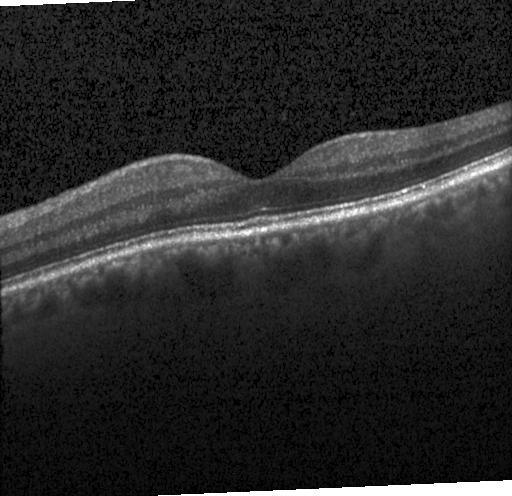
Heidelberg Spectralis. Optical coherence tomography B-scan. Dx: no choroidal neovascularization, diabetic macular edema, or drusen.